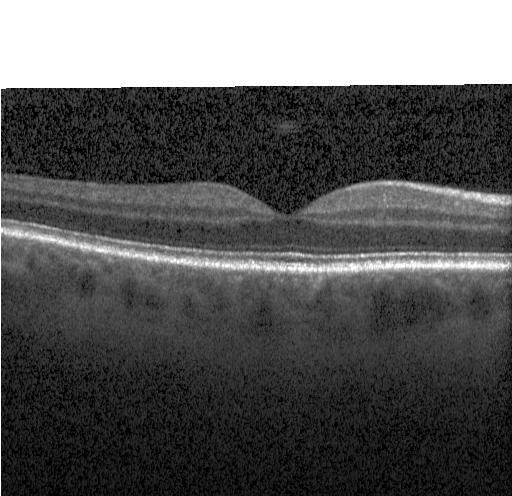

Optical coherence tomography scan. Through the macula. Acquired on a Heidelberg Spectralis. Spectral-domain optical coherence tomography.
Assessment: neither CNV, DME, nor drusen.